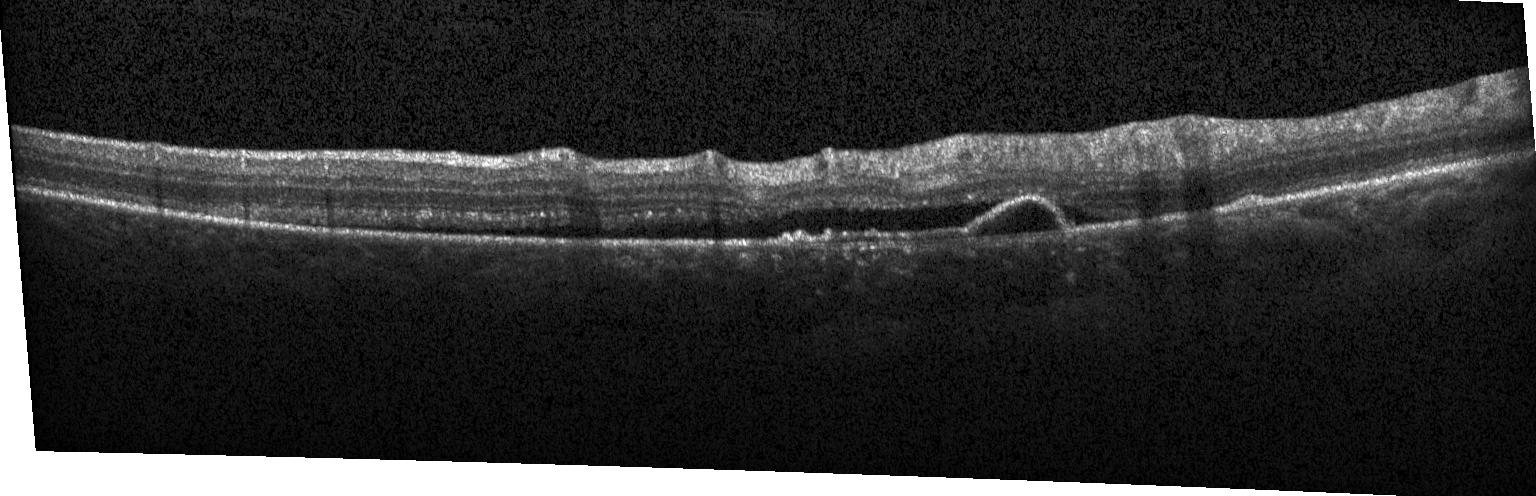 OCT B-scan showing choroidal neovascularization (CNV).